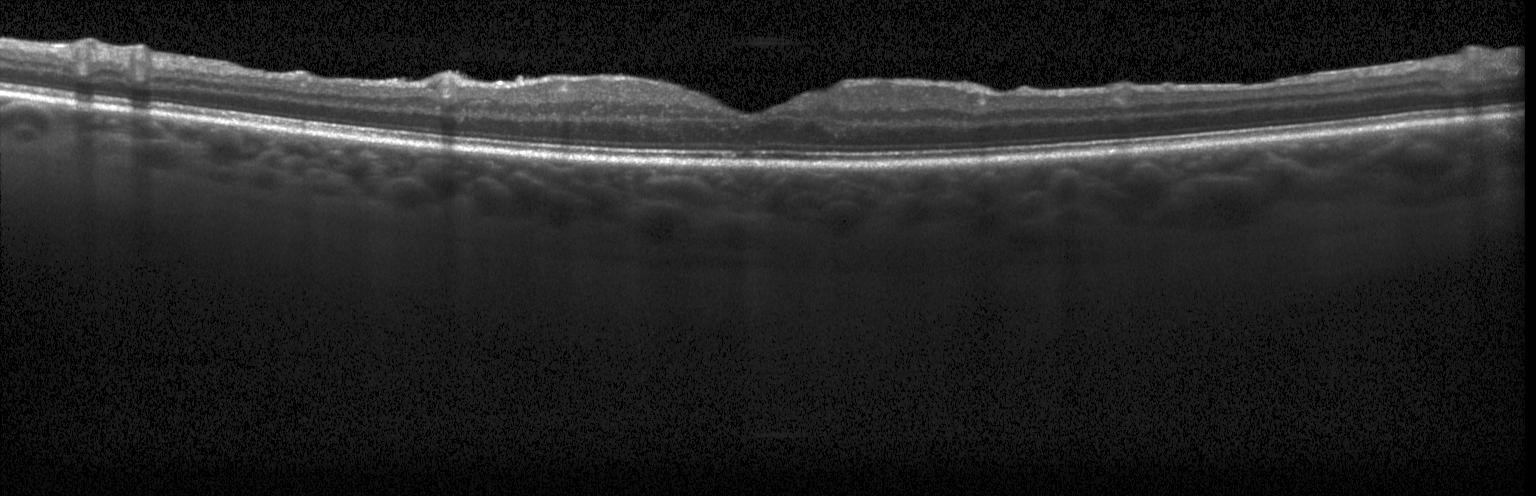
Spectral-domain OCT; acquired on a Heidelberg Spectralis; through the macula; optical coherence tomography B-scan
Finding: no choroidal neovascularization, diabetic macular edema, or drusen.